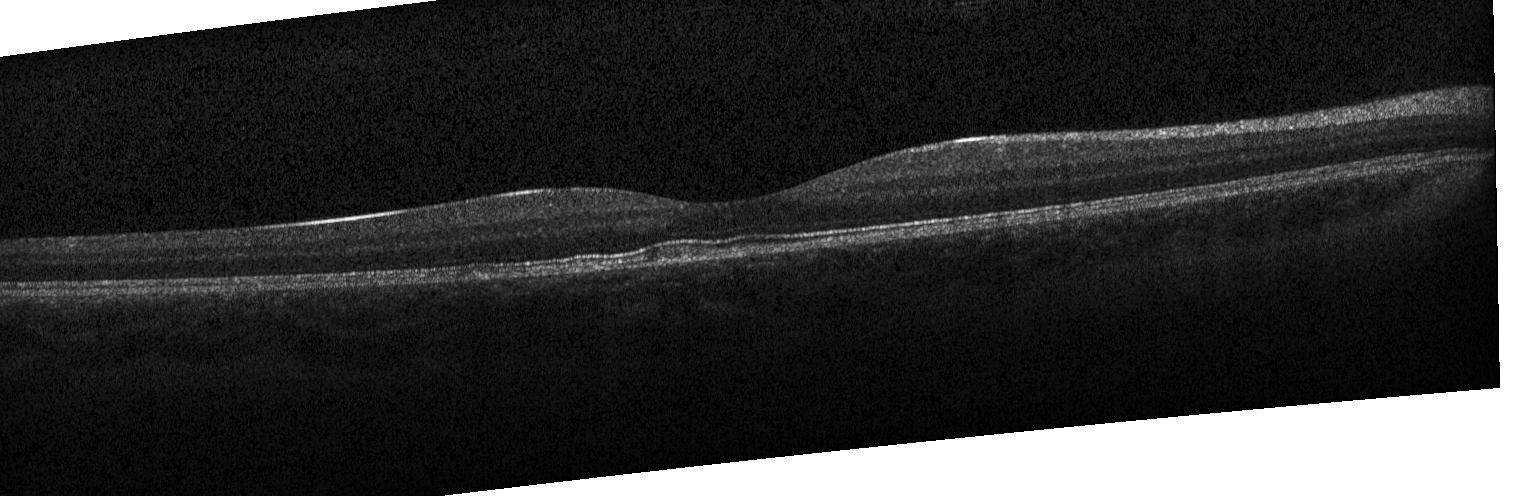 Horizontal scan through the fovea. Retinal OCT B-scan. Spectral-domain OCT — Finding: no choroidal neovascularization, no diabetic macular edema, and no drusen.